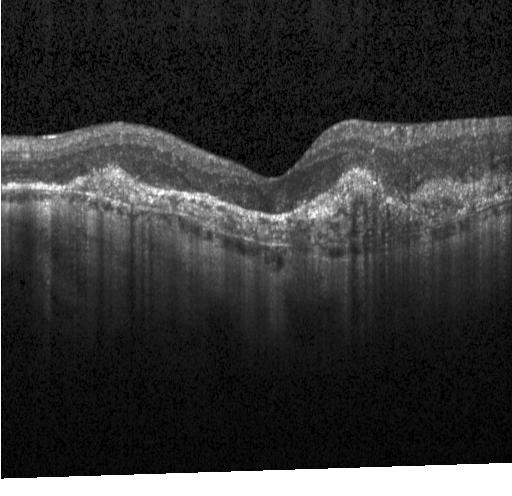

CNV.